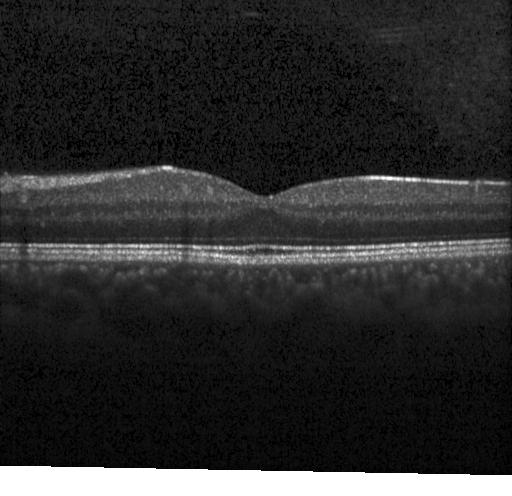

Diagnosis: no CNV, DME, or drusen.